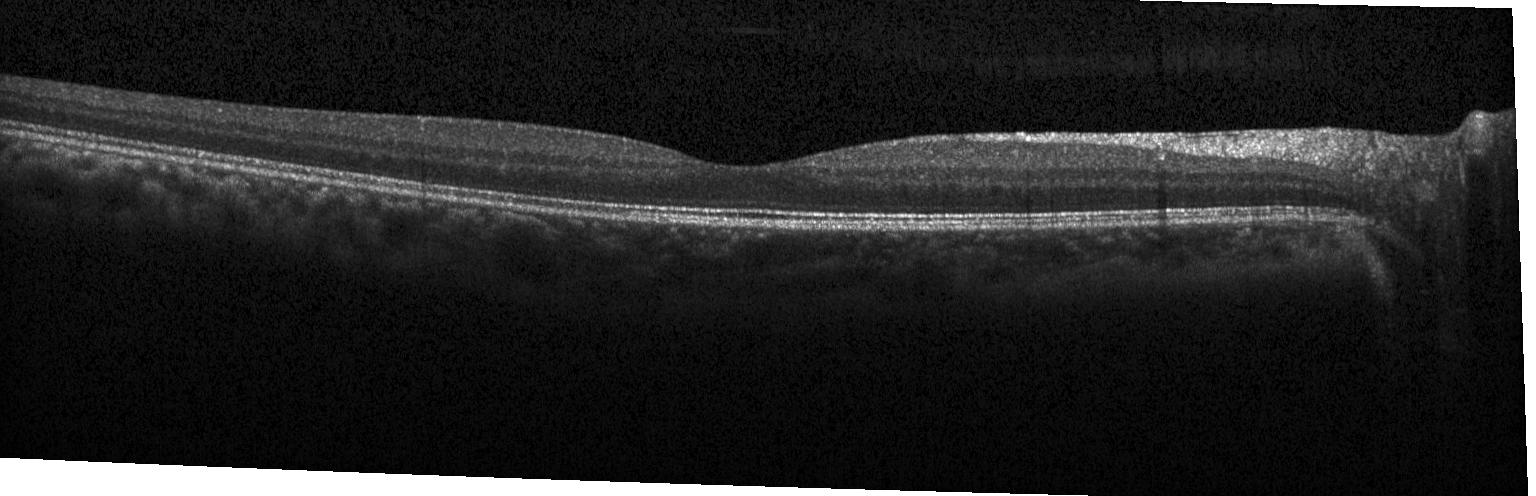 OCT line scan · spectral-domain OCT.
Impression: no choroidal neovascularization, no diabetic macular edema, and no drusen.